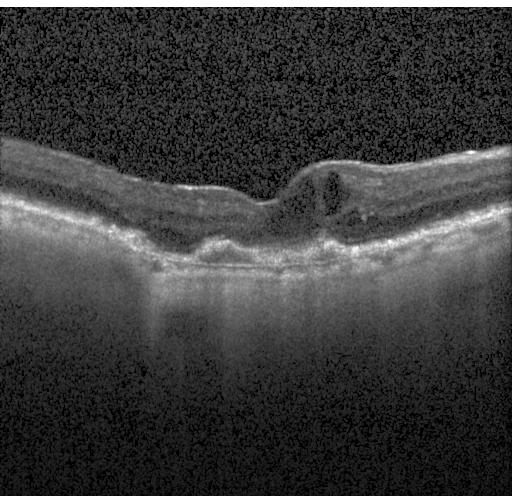 OCT B-scan showing CNV.